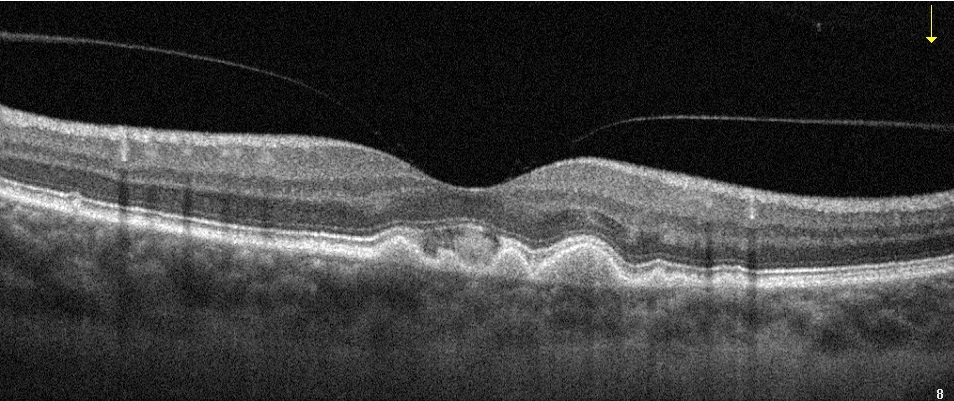

OCT line scan, fovea-centered
Diagnosis: age-related macular degeneration.